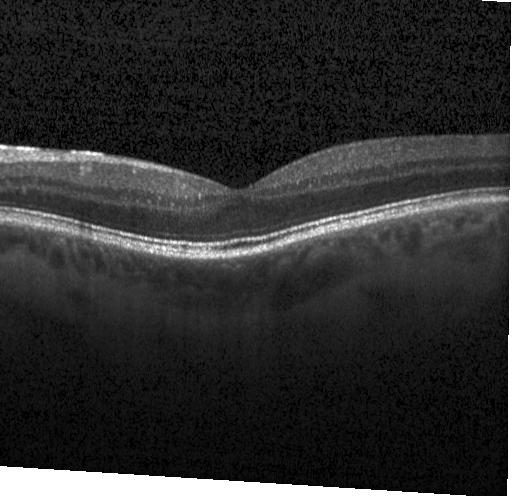
Macular scan. Heidelberg Spectralis. OCT B-scan. SD-OCT
Assessment: neither choroidal neovascularization, diabetic macular edema, nor drusen.